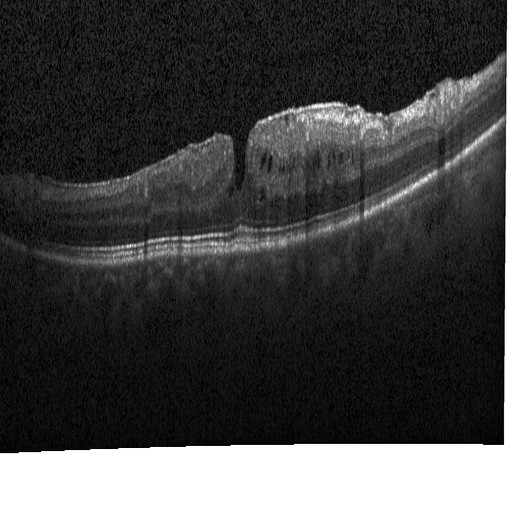
Optical coherence tomography B-scan · instrument: Heidelberg Spectralis. OCT finding: diabetic macular edema (DME).